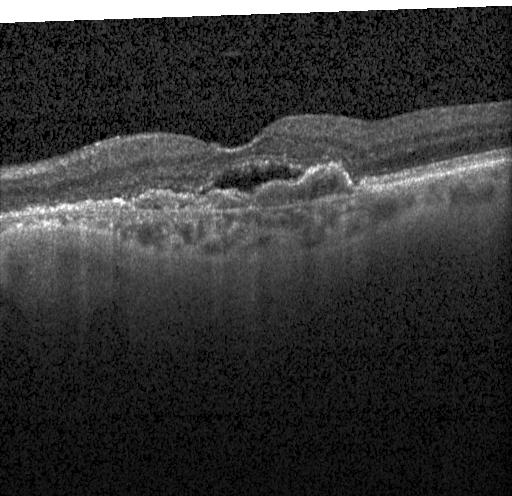 Optical coherence tomography scan, Heidelberg Spectralis OCT system, centered on the fovea
Finding: CNV.